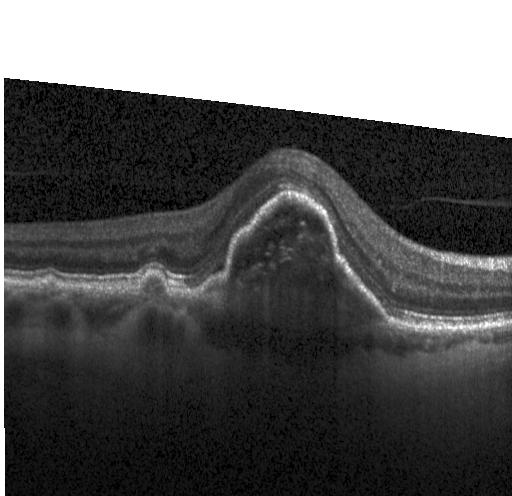 A choroidal neovascular membrane.